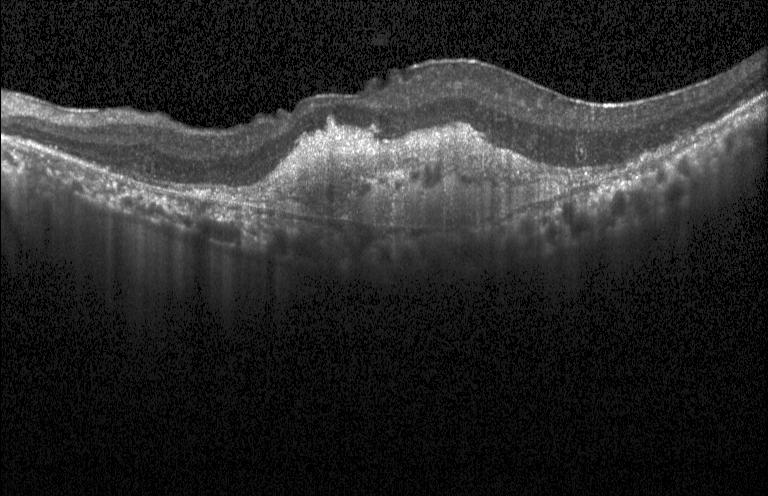
Macular OCT: CNV.